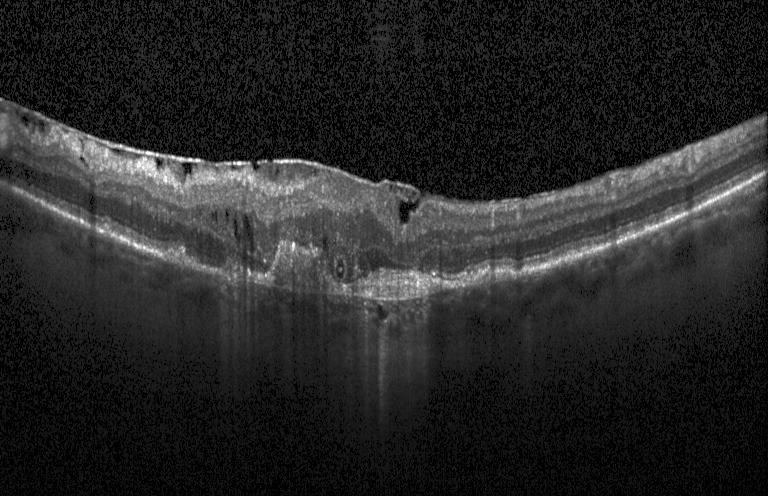
OCT line scan — Finding: choroidal neovascularization.